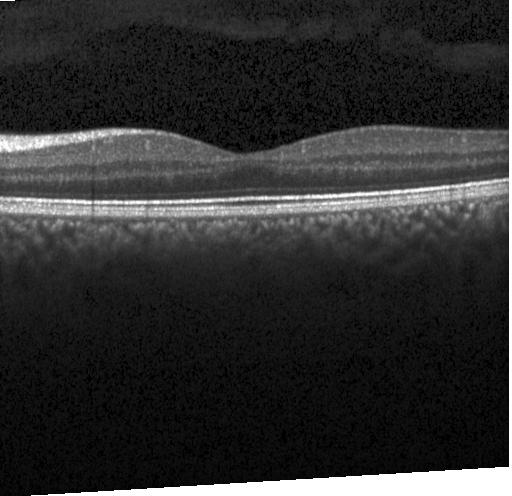
OCT finding: no choroidal neovascularization, no diabetic macular edema, and no drusen.